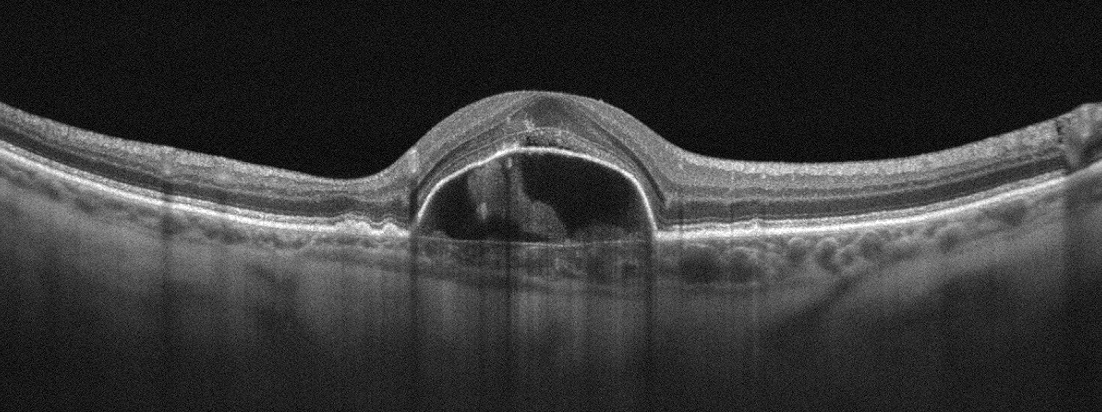

OCT B-scan showing age-related macular degeneration (AMD).